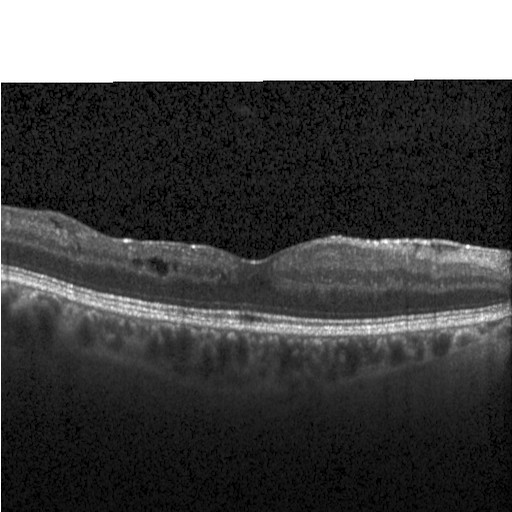 Diabetic macular edema (DME).